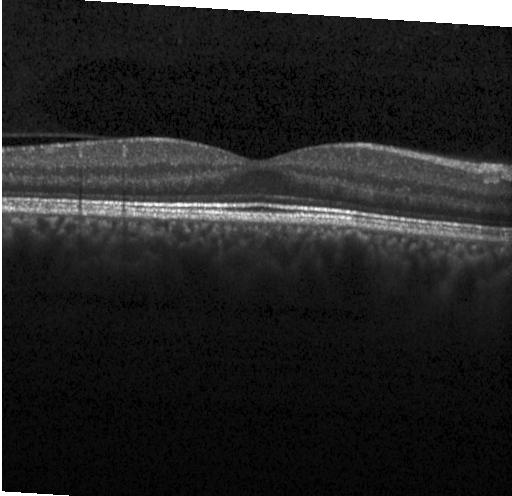 Retinal OCT cross-section showing no evidence of choroidal neovascularization, diabetic macular edema, or drusen.